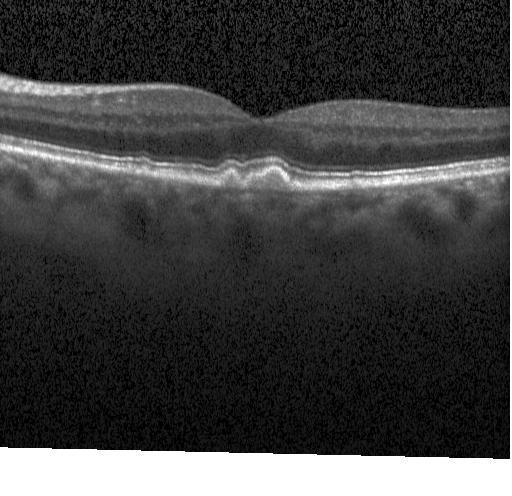
Optical coherence tomography scan · SD-OCT · acquired on a Heidelberg Spectralis — This B-scan demonstrates sub-RPE drusenoid deposits.